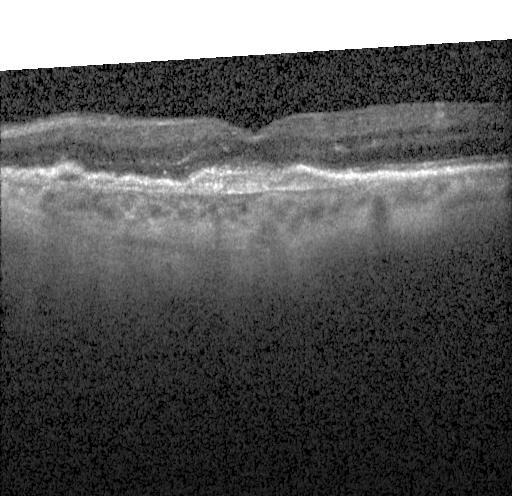 Optical coherence tomography scan. A choroidal neovascular membrane.